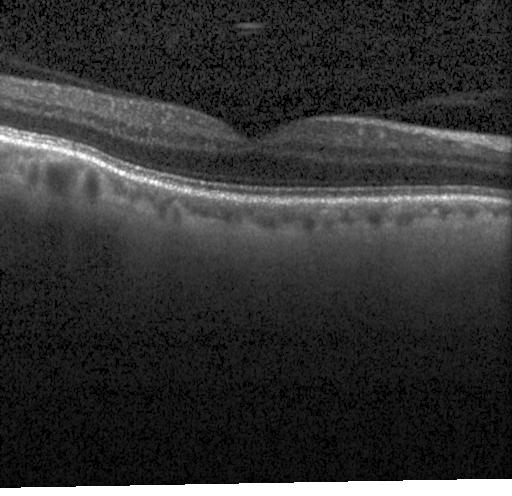 Retinal OCT B-scan — Diagnosis: no choroidal neovascularization, no diabetic macular edema, and no drusen.